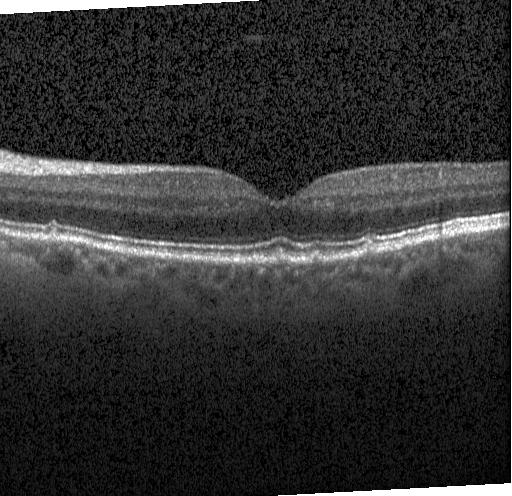 Spectral-domain optical coherence tomography. OCT line scan. Acquired on a Heidelberg Spectralis. Fovea-centered.
Impression: sub-RPE drusenoid deposits.